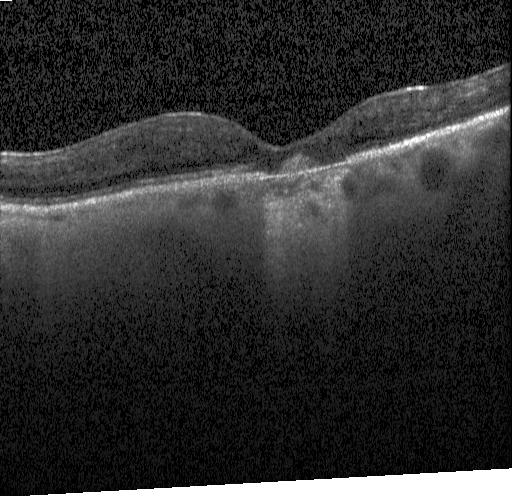

Retinal OCT B-scan. Centered on the fovea. Acquired on a Heidelberg Spectralis
Dx: a choroidal neovascular membrane.